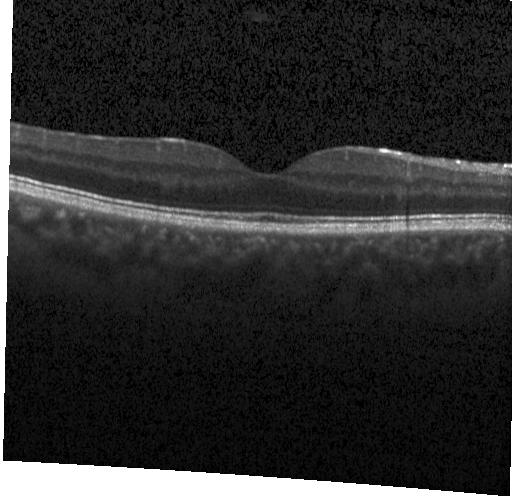
Fovea-centered, retinal OCT B-scan, Heidelberg Spectralis OCT system, spectral-domain optical coherence tomography
The scan shows neither choroidal neovascularization, diabetic macular edema, nor drusen.